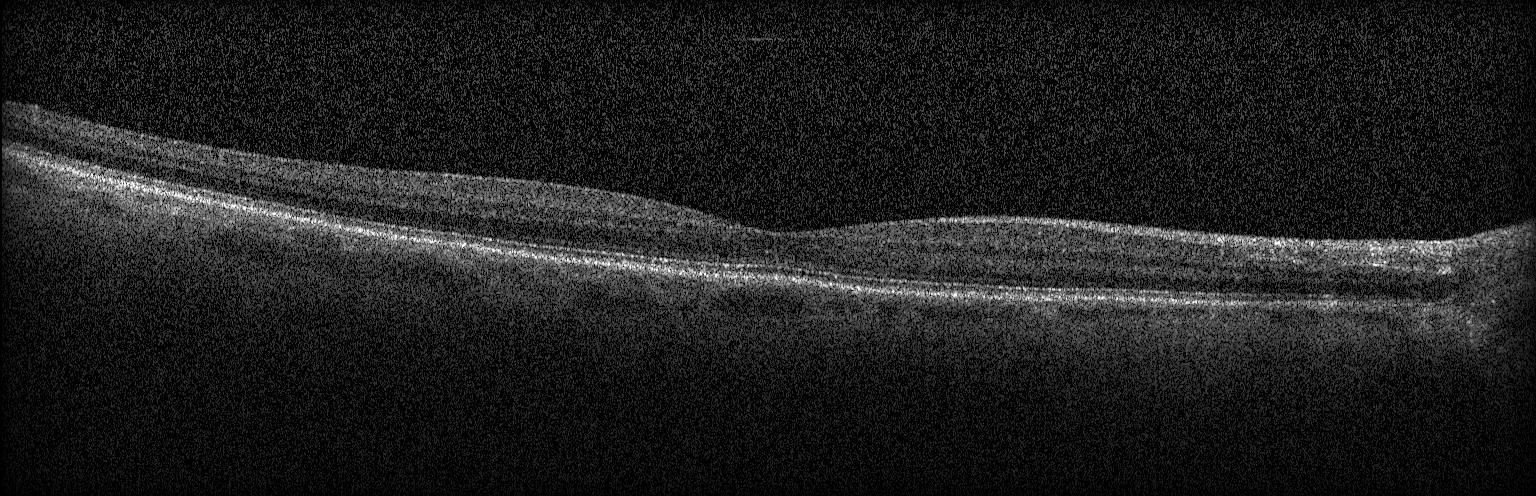

Diagnosis: no choroidal neovascularization, no diabetic macular edema, and no drusen.